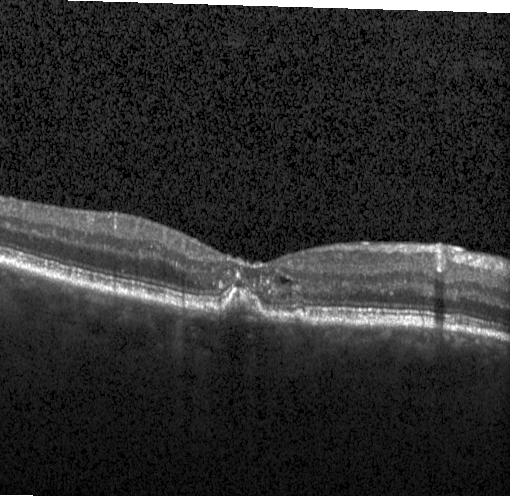 A choroidal neovascular membrane.